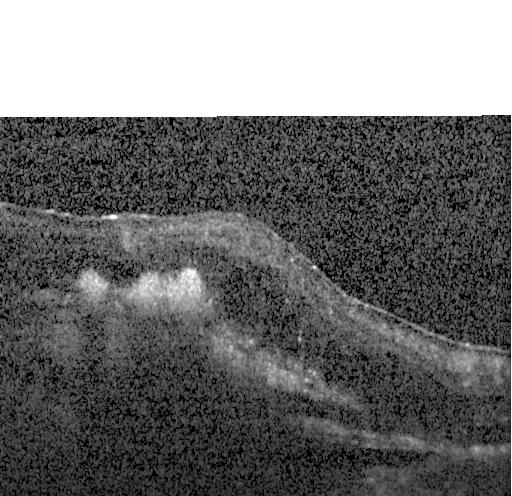
Optical coherence tomography scan, horizontal scan through the fovea, acquired on a Heidelberg Spectralis. A choroidal neovascular membrane.